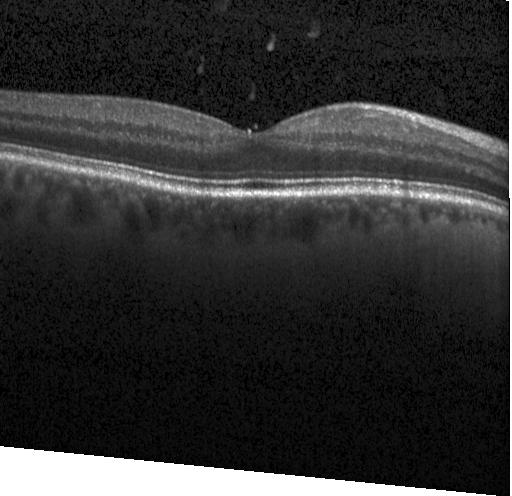 SD-OCT · OCT line scan · acquired on a Heidelberg Spectralis · macular scan — This B-scan demonstrates no choroidal neovascularization, diabetic macular edema, or drusen.